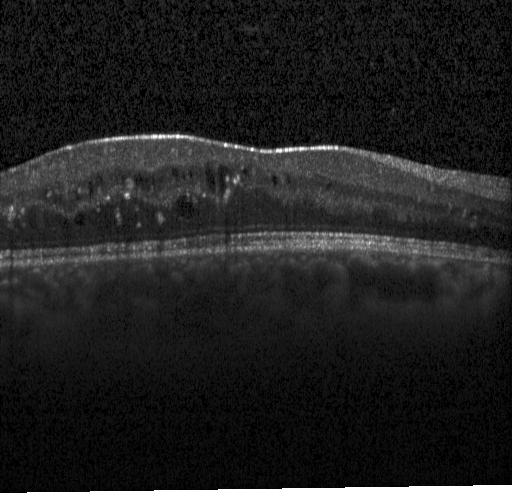 Macular scan; retinal OCT B-scan; Heidelberg Spectralis.
DME.